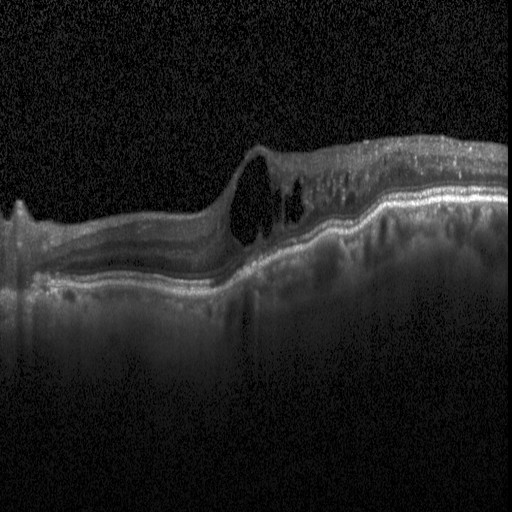 OCT finding: diabetic macular edema (DME).